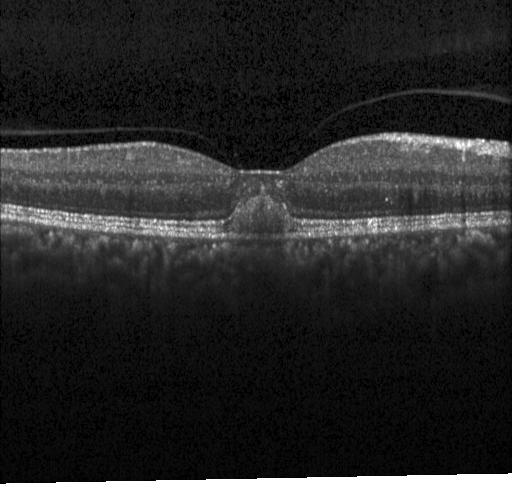

Spectral-domain optical coherence tomography. Acquired on a Heidelberg Spectralis. Centered on the fovea. OCT line scan. This B-scan demonstrates a choroidal neovascular membrane.